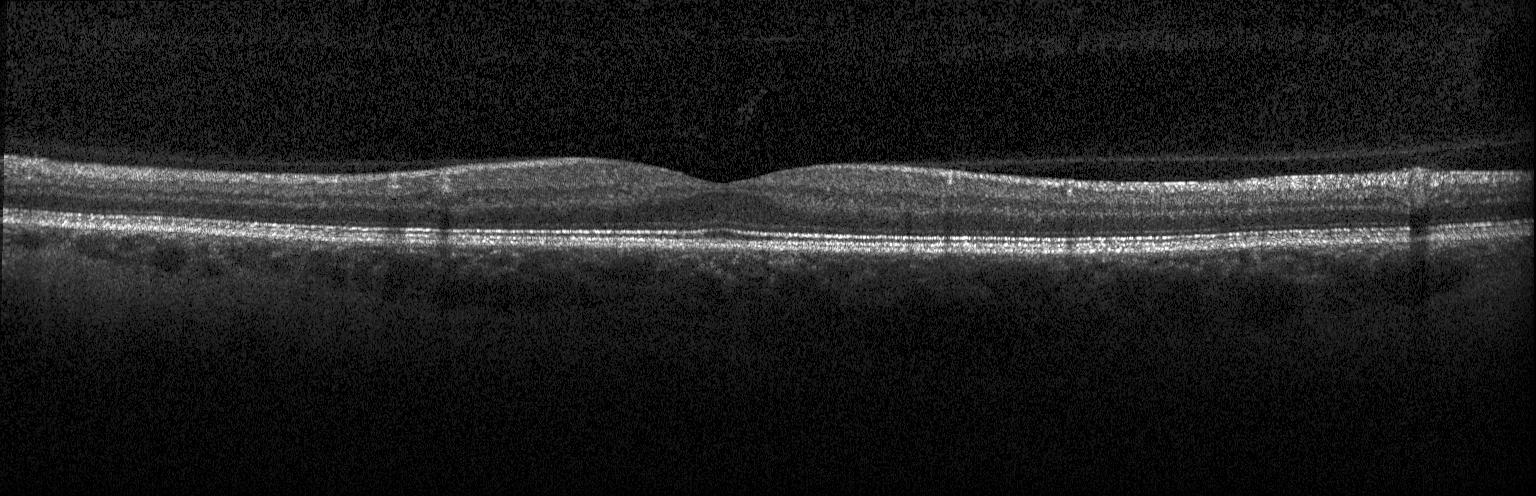
Through the macula, optical coherence tomography scan, spectral-domain optical coherence tomography
Impression: no CNV, DME, or drusen.